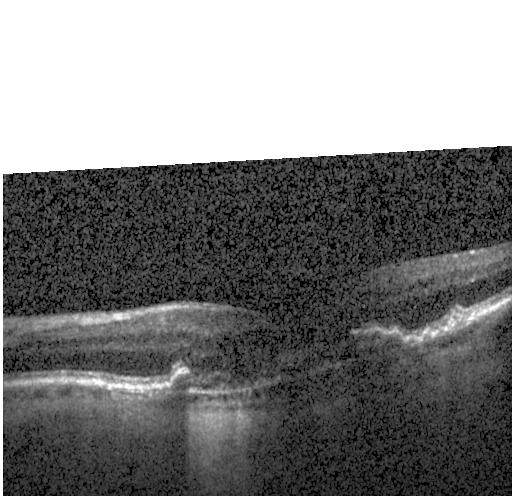
Spectral-domain optical coherence tomography. Optical coherence tomography B-scan.
Choroidal neovascularization (CNV).